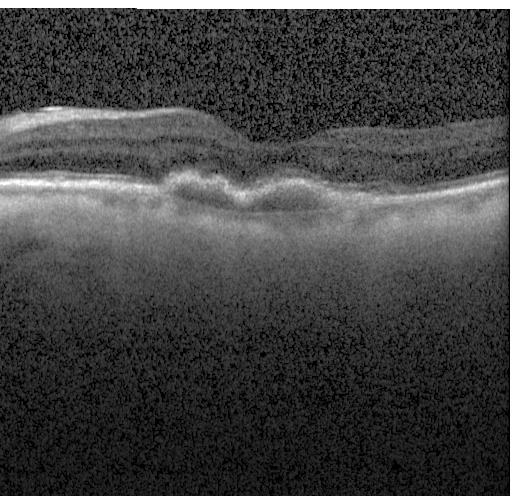

Optical coherence tomography scan, instrument: Heidelberg Spectralis, SD-OCT — Assessment: choroidal neovascularization (CNV).